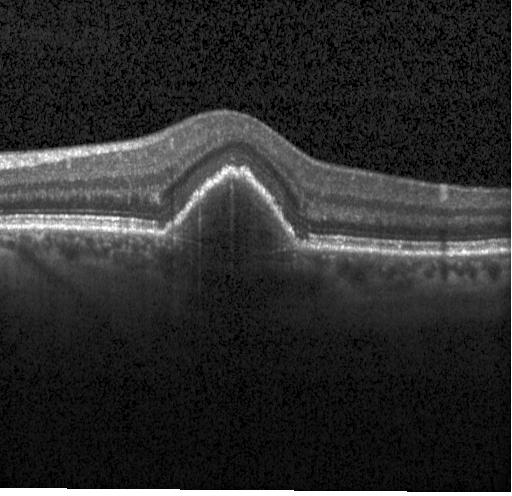
Macular OCT: a choroidal neovascular membrane.